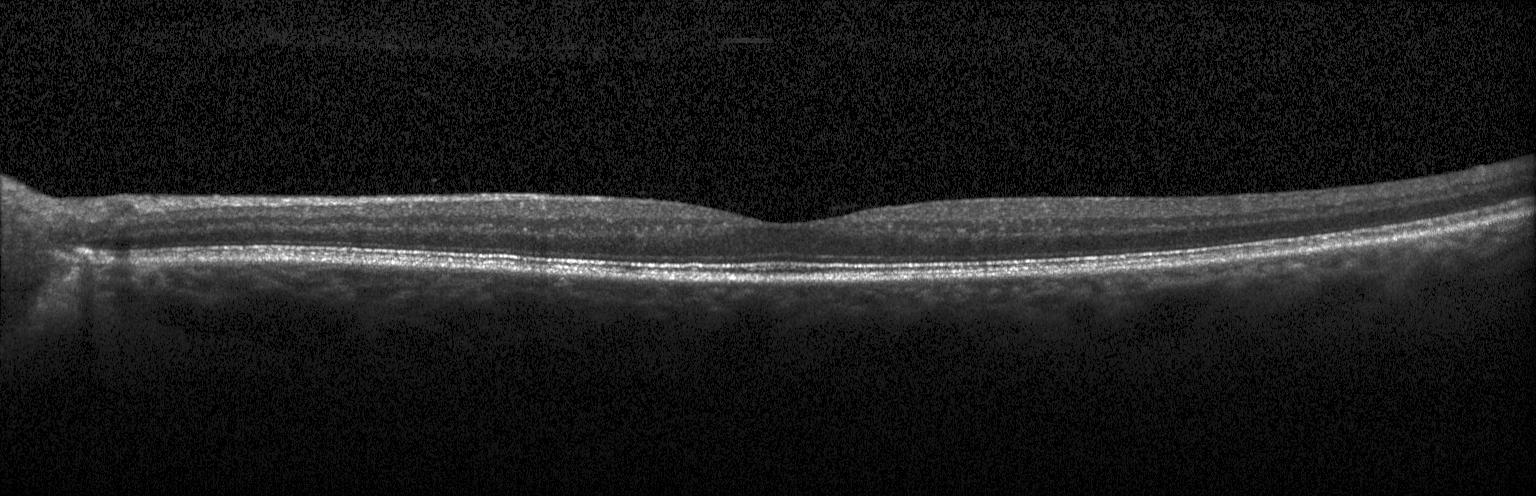
Spectral-domain OCT · Heidelberg Spectralis · optical coherence tomography scan · centered on the fovea — Neither choroidal neovascularization, diabetic macular edema, nor drusen.